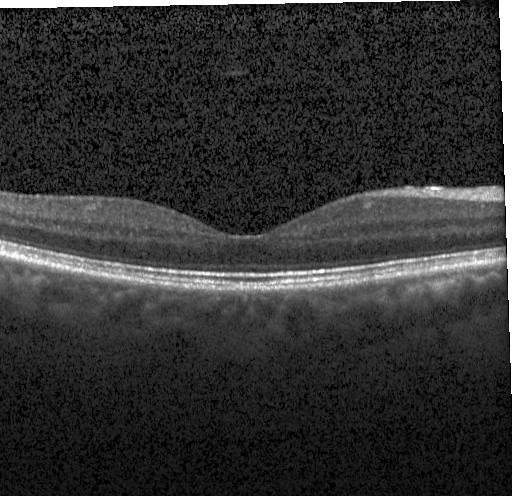
Macular OCT: no choroidal neovascularization, diabetic macular edema, or drusen.